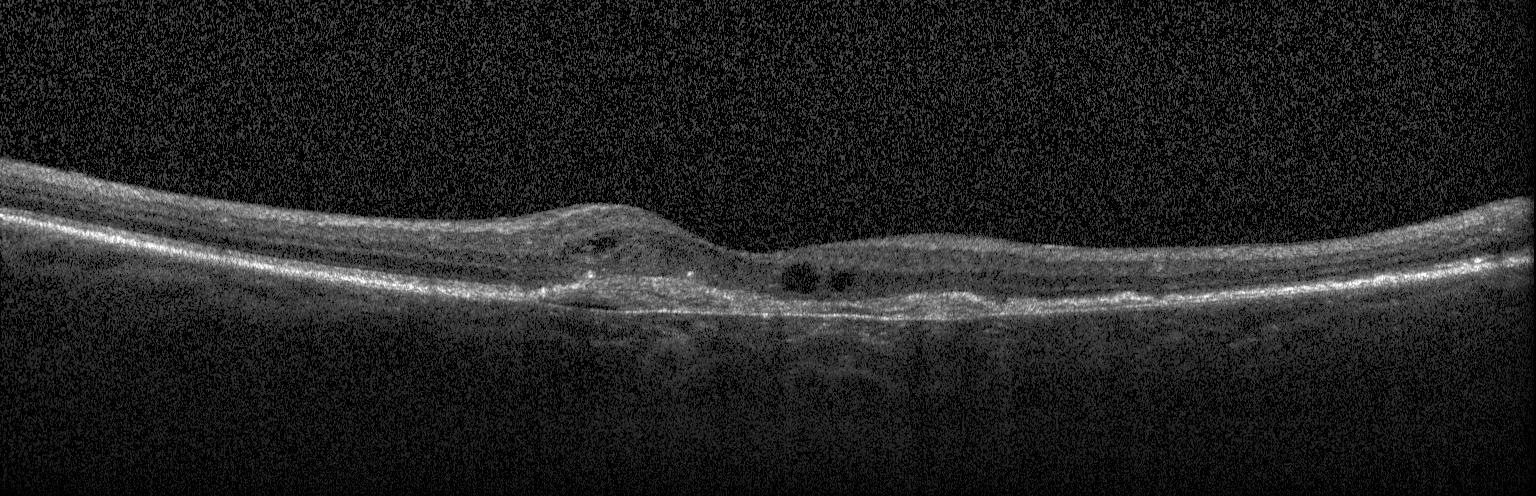
Optical coherence tomography B-scan; acquired on a Heidelberg Spectralis; horizontal scan through the fovea.
Assessment: choroidal neovascularization (CNV).